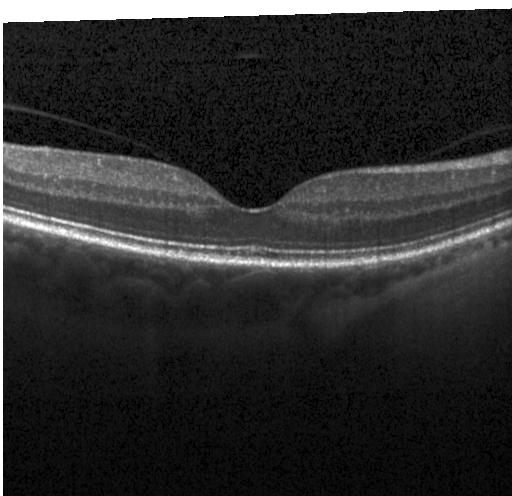
Macular OCT: no evidence of choroidal neovascularization, diabetic macular edema, or drusen.